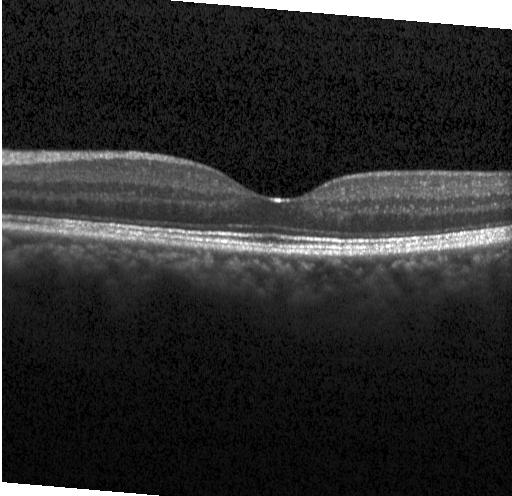 Diagnosis: no CNV, no DME, and no drusen.